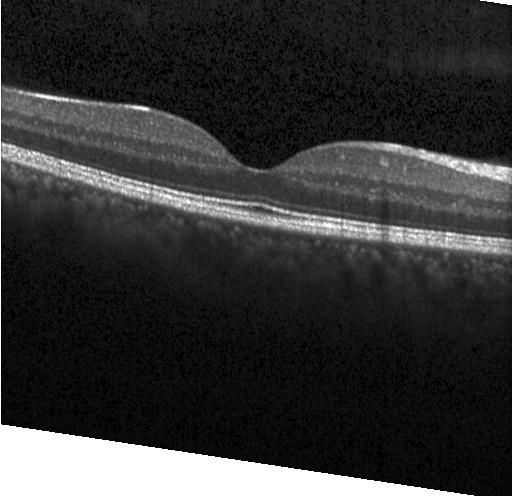

OCT scan showing no choroidal neovascularization, diabetic macular edema, or drusen.